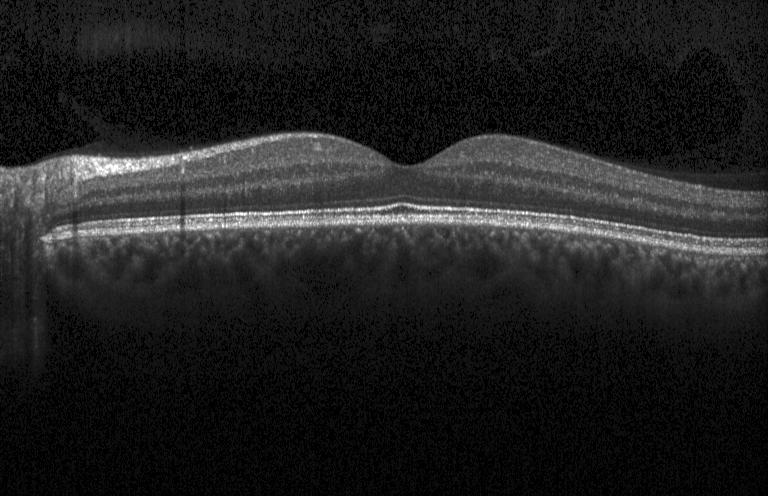
Retinal OCT B-scan.
Dx: neither choroidal neovascularization, diabetic macular edema, nor drusen.